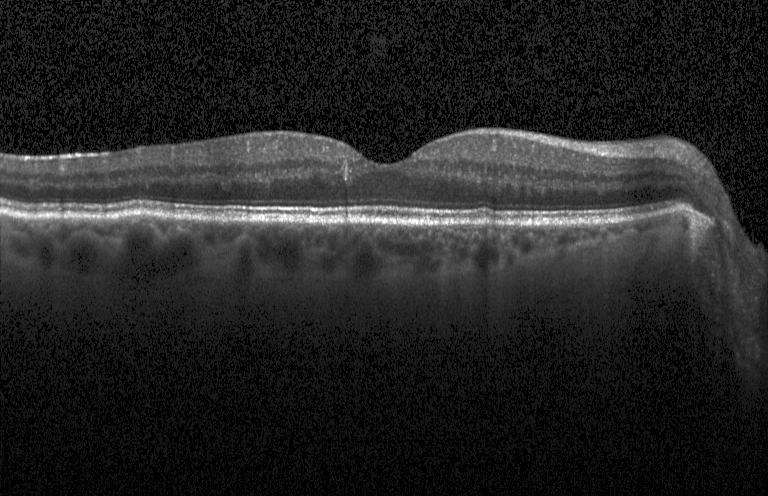 Spectral-domain OCT B-scan: no evidence of CNV, DME, or drusen.